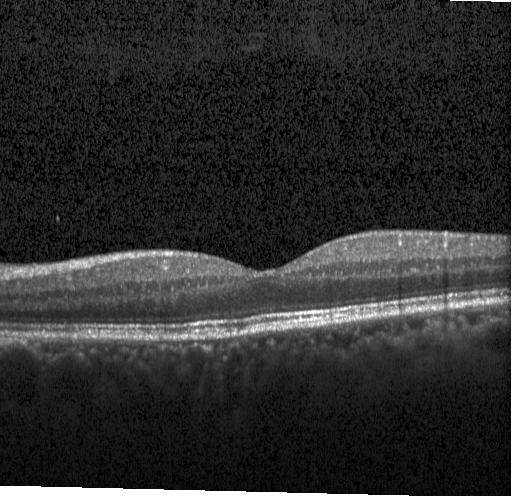 Dx: no evidence of choroidal neovascularization, diabetic macular edema, or drusen.